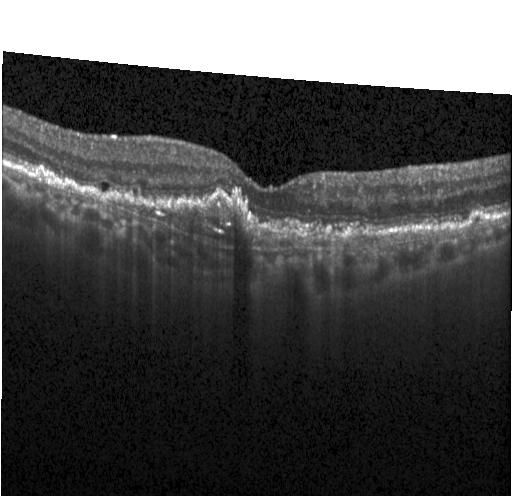

OCT finding: CNV.